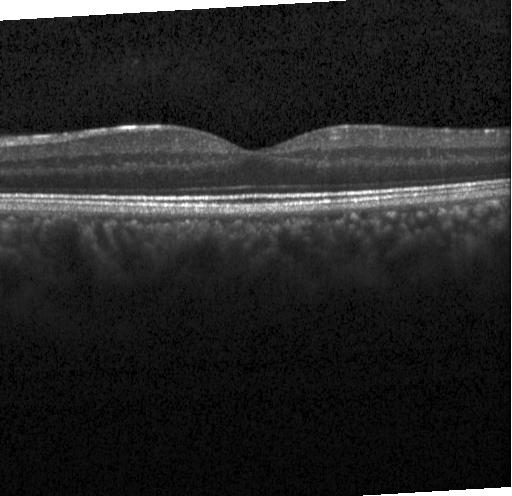 Retinal OCT cross-section · spectral-domain optical coherence tomography.
Finding: no CNV, no DME, and no drusen.